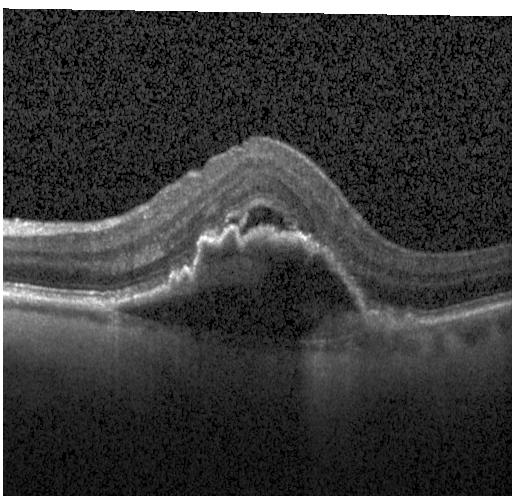

Macular OCT: a choroidal neovascular membrane.